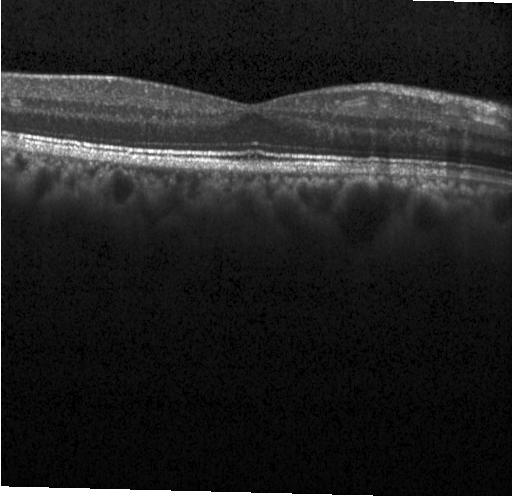

Macular OCT: no CNV, DME, or drusen.